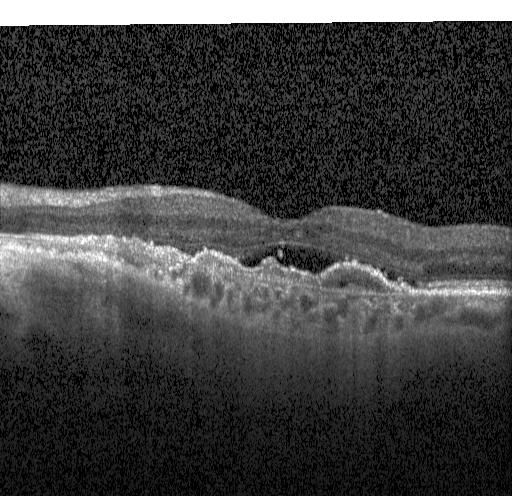 Impression: a choroidal neovascular membrane.